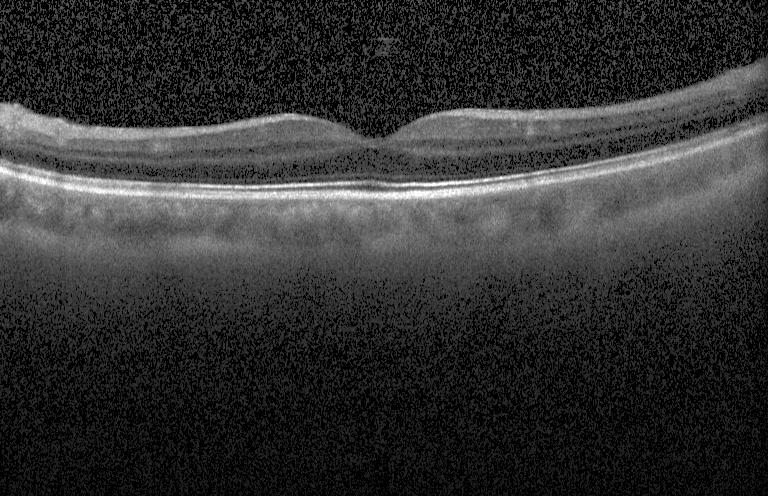
OCT B-scan showing no choroidal neovascularization, diabetic macular edema, or drusen.